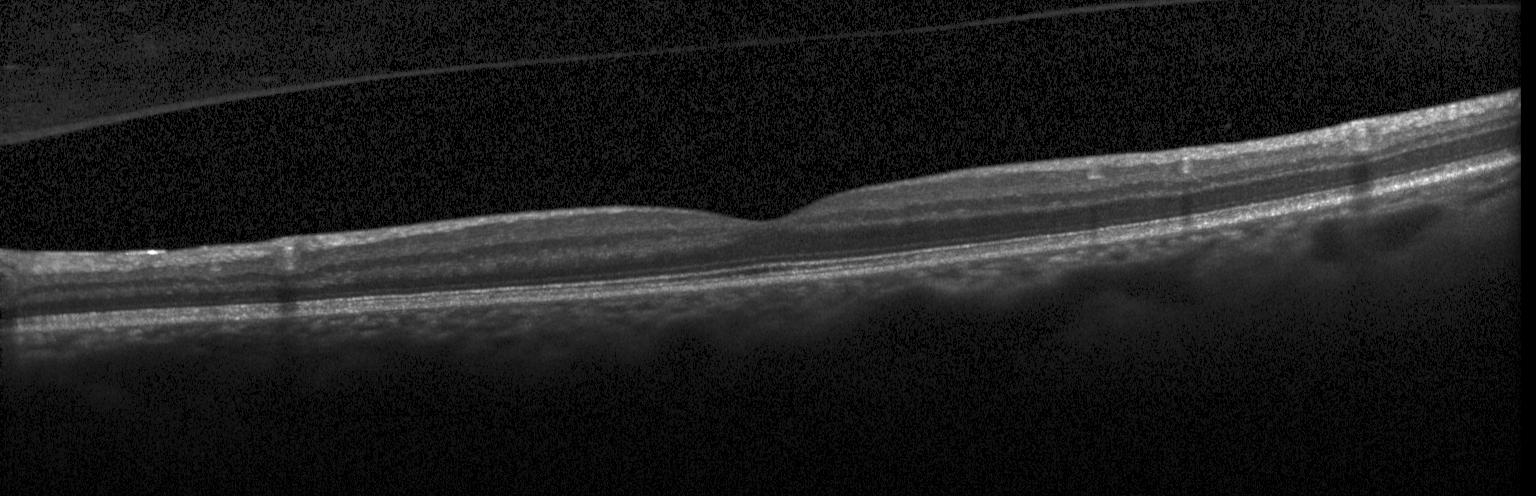

Centered on the fovea, optical coherence tomography scan, acquired on a Heidelberg Spectralis
Impression: no evidence of choroidal neovascularization, diabetic macular edema, or drusen.